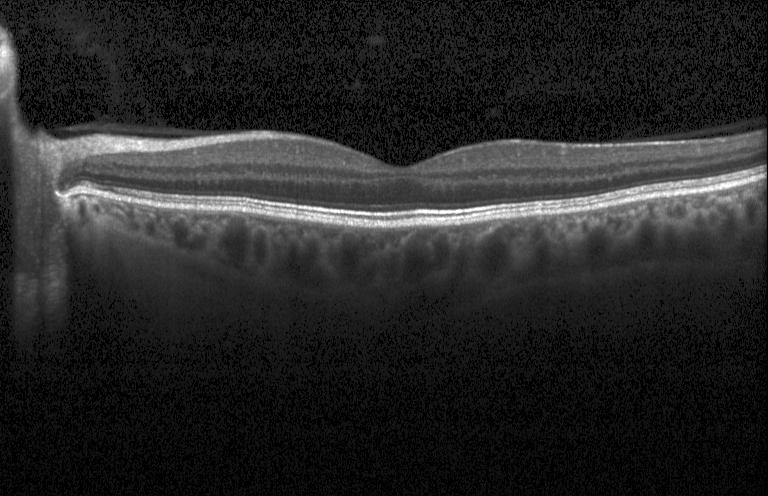

Instrument: Heidelberg Spectralis; optical coherence tomography scan; spectral-domain OCT.
This B-scan demonstrates no evidence of CNV, DME, or drusen.